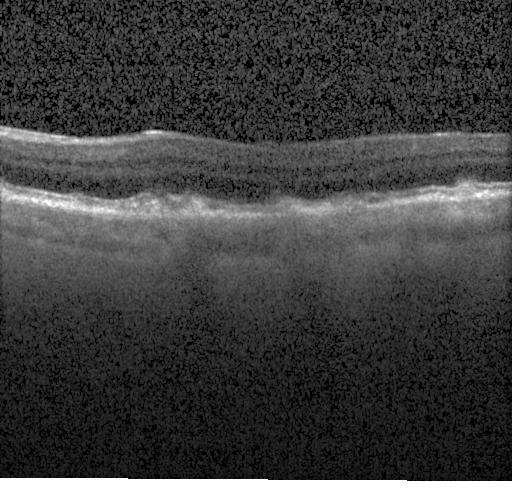
OCT line scan. This B-scan demonstrates drusen.